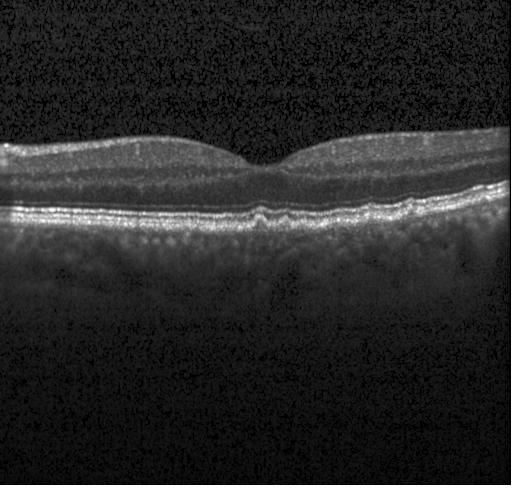

Macular OCT demonstrating multiple drusen.